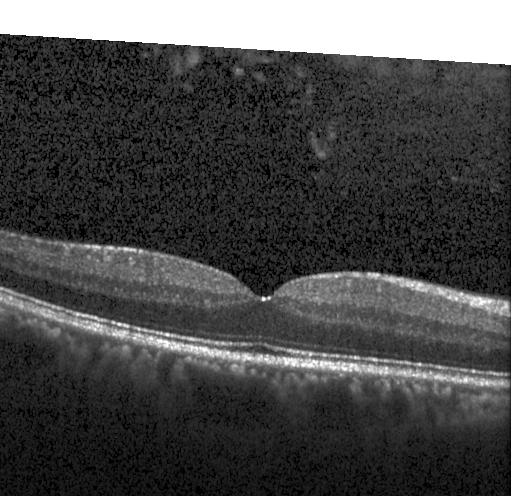 Finding: no CNV, no DME, and no drusen.